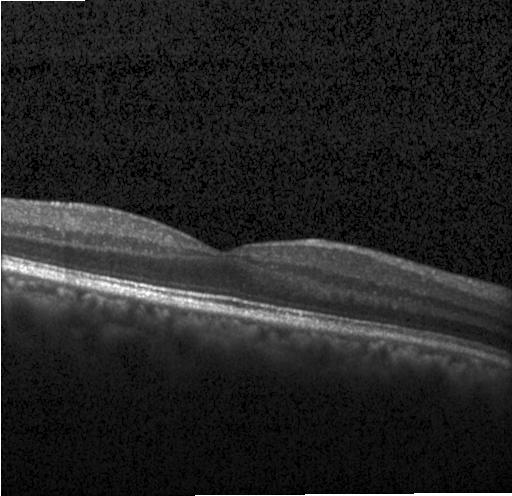 OCT finding: no evidence of choroidal neovascularization, diabetic macular edema, or drusen.